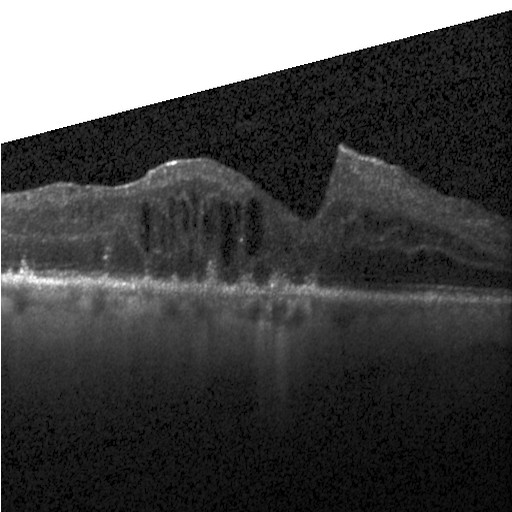 Dx: diabetic macular edema (DME).